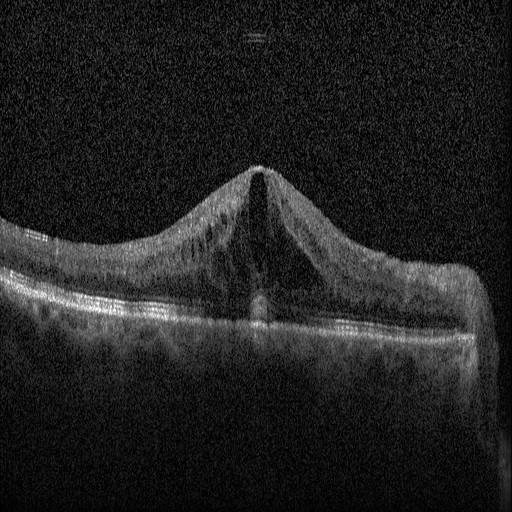

Fovea-centered, instrument: Heidelberg Spectralis, SD-OCT, retinal OCT cross-section.
Diagnosis: DME.